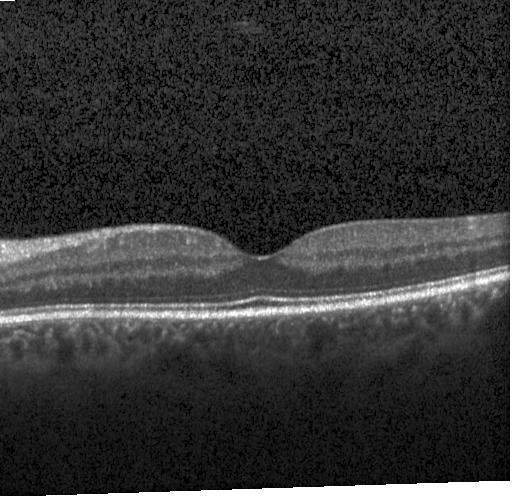 Macular scan; OCT line scan — Diagnosis: no choroidal neovascularization, no diabetic macular edema, and no drusen.